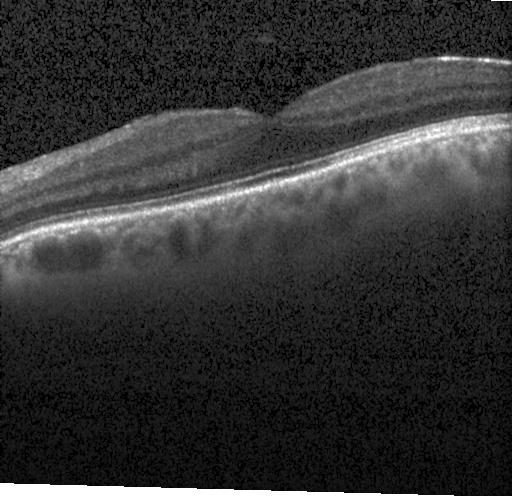 Centered on the fovea · Heidelberg Spectralis · OCT B-scan.
OCT finding: neither CNV, DME, nor drusen.